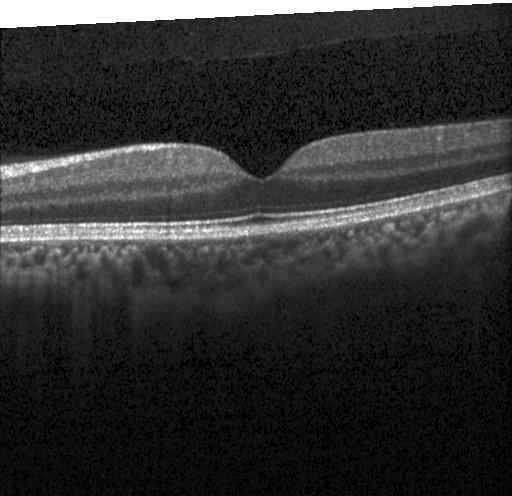 Optical coherence tomography scan; spectral-domain optical coherence tomography; Heidelberg Spectralis
The scan shows neither choroidal neovascularization, diabetic macular edema, nor drusen.